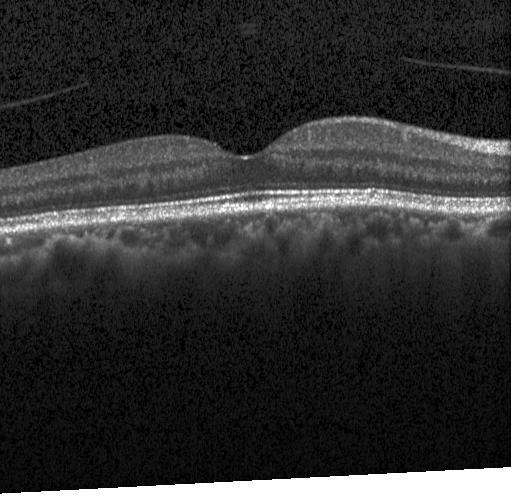 Impression: neither CNV, DME, nor drusen.